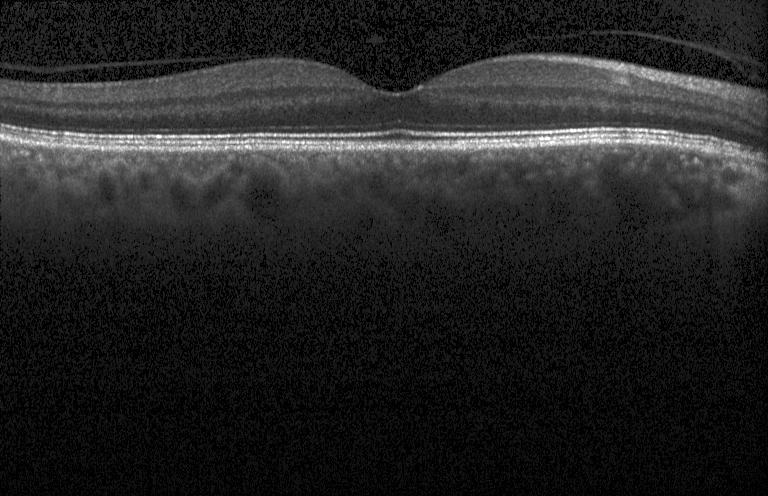 Retinal OCT cross-section; through the macula; Heidelberg Spectralis OCT system — Dx: neither choroidal neovascularization, diabetic macular edema, nor drusen.